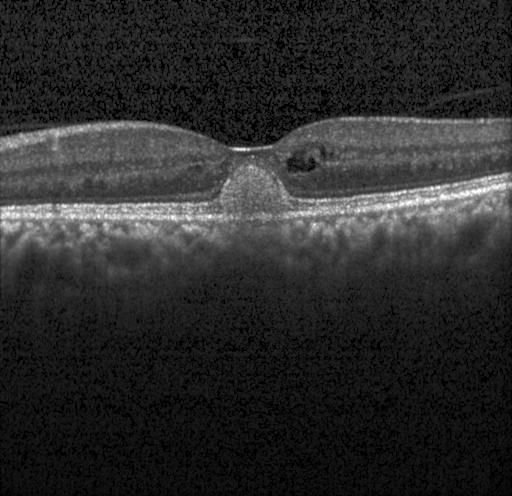
Diagnosis: choroidal neovascularization (CNV).